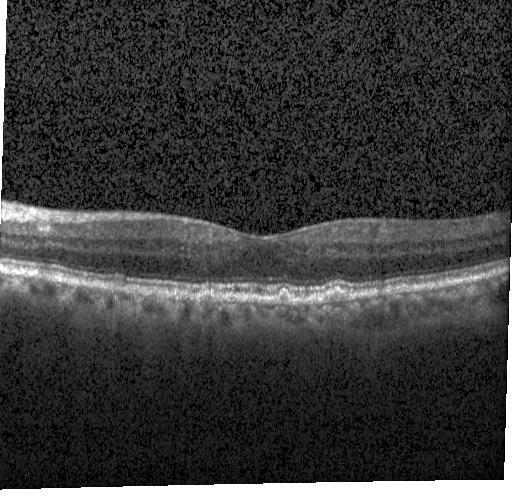

Optical coherence tomography B-scan. The scan shows drusen.